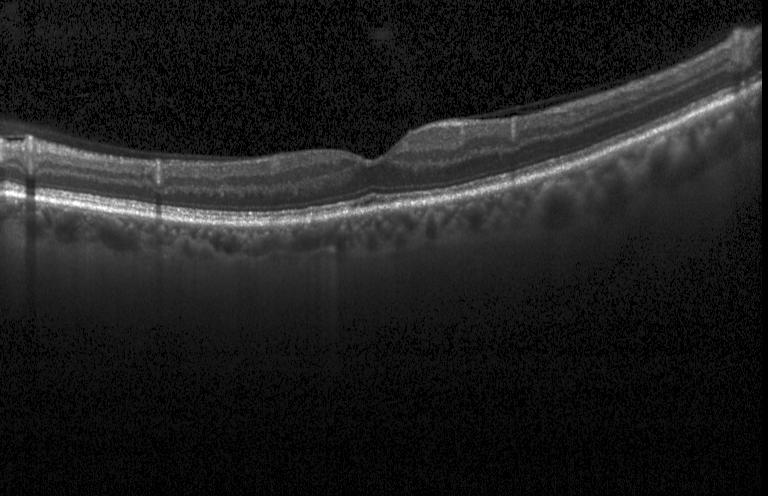
OCT B-scan. Macular scan. Impression: no evidence of choroidal neovascularization, diabetic macular edema, or drusen.